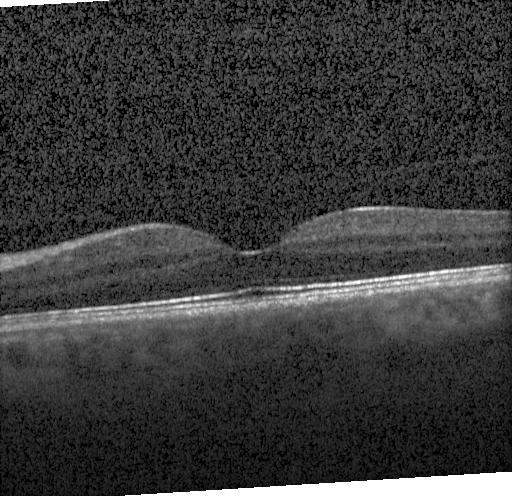 Retinal OCT cross-section showing no evidence of CNV, DME, or drusen.